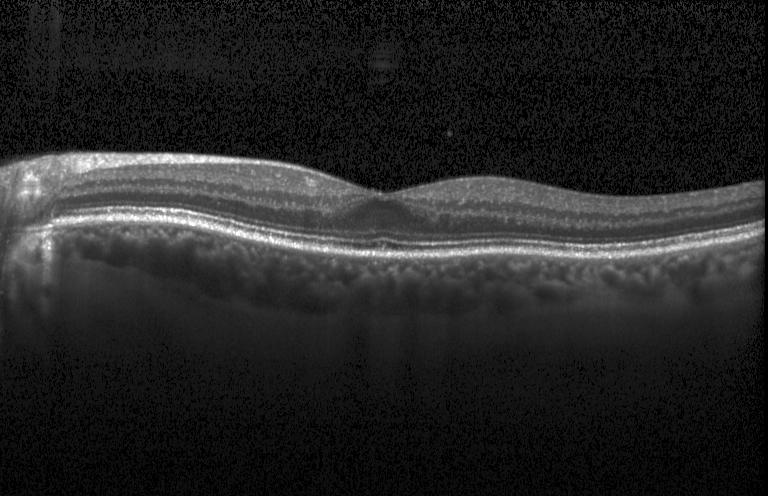

OCT line scan.
Assessment: no choroidal neovascularization, diabetic macular edema, or drusen.